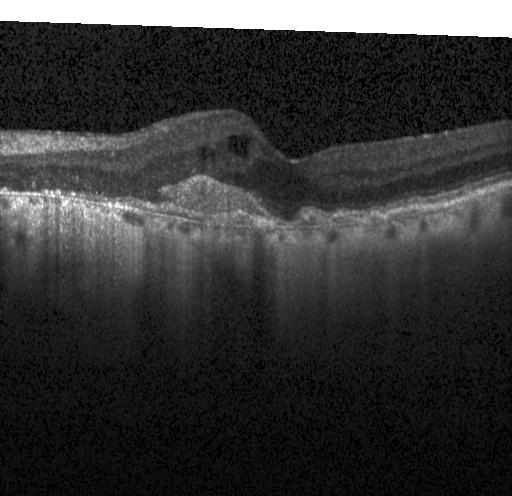 Macular OCT: choroidal neovascularization (CNV).